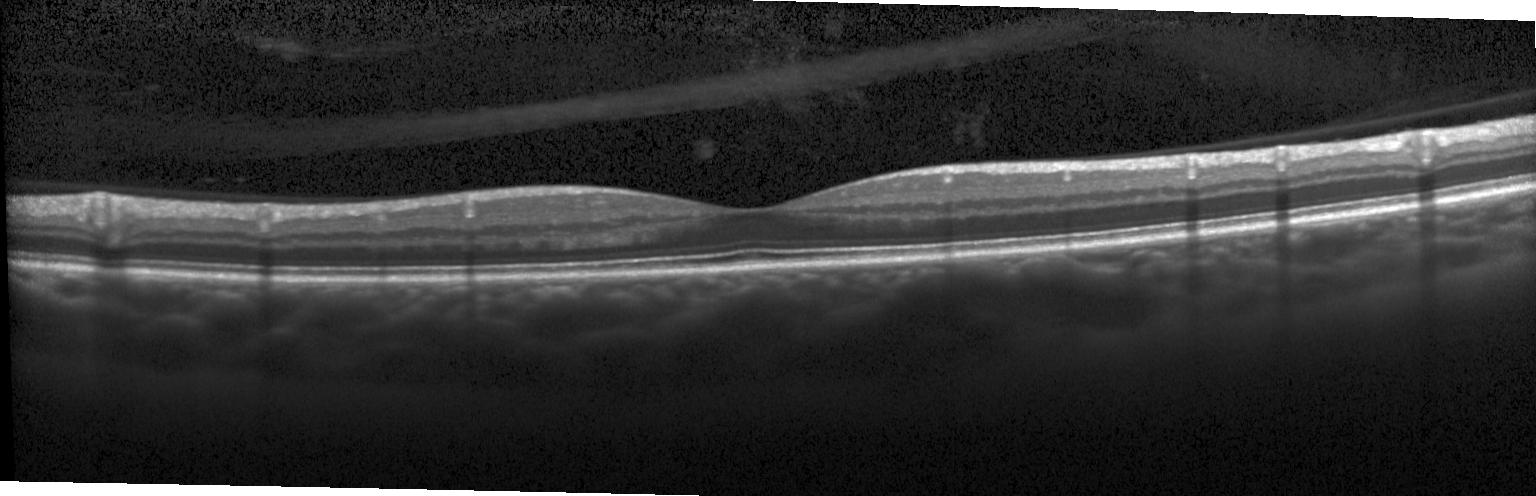
Retinal OCT cross-section; through the macula; spectral-domain optical coherence tomography
Diagnosis: no CNV, DME, or drusen.